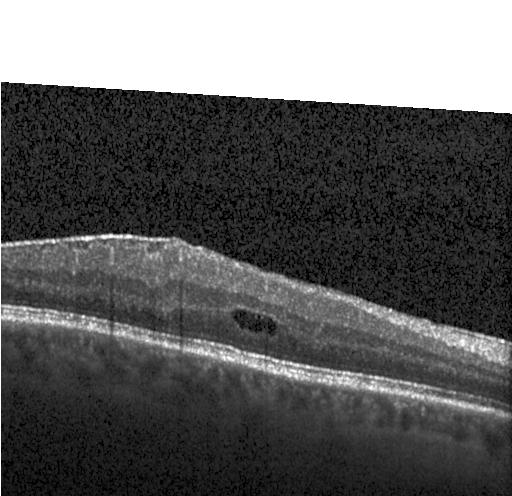

Macular scan; spectral-domain OCT; OCT B-scan; Heidelberg Spectralis — This B-scan demonstrates diabetic macular edema.